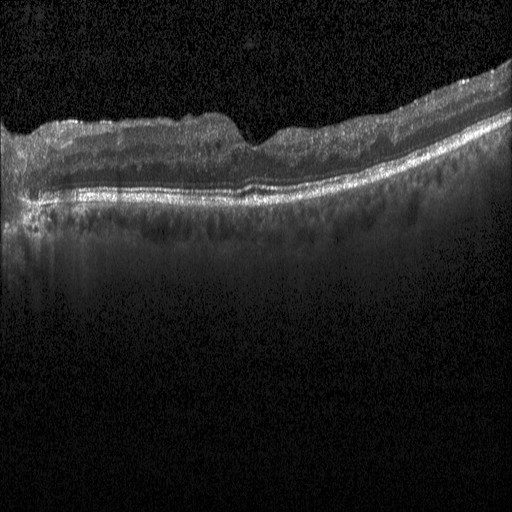 Optical coherence tomography scan. Acquired on a Heidelberg Spectralis. Fovea-centered. SD-OCT.
Diagnosis: diabetic macular edema (DME).